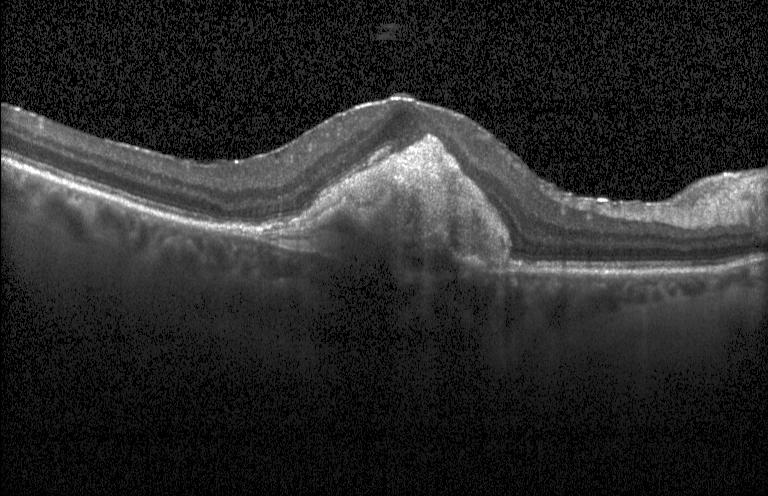
Retinal OCT cross-section. Acquired on a Heidelberg Spectralis. A choroidal neovascular membrane.